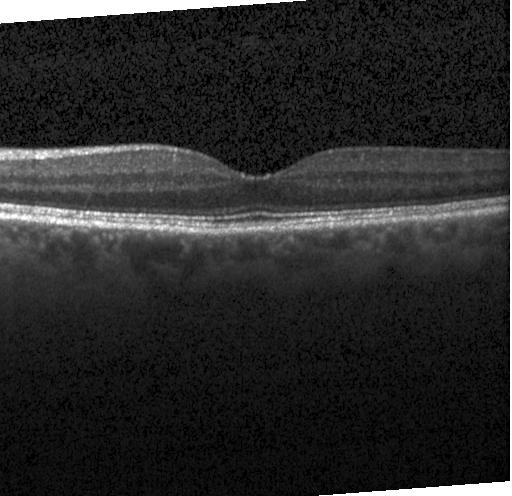

Fovea-centered. Retinal OCT B-scan
No CNV, no DME, and no drusen.